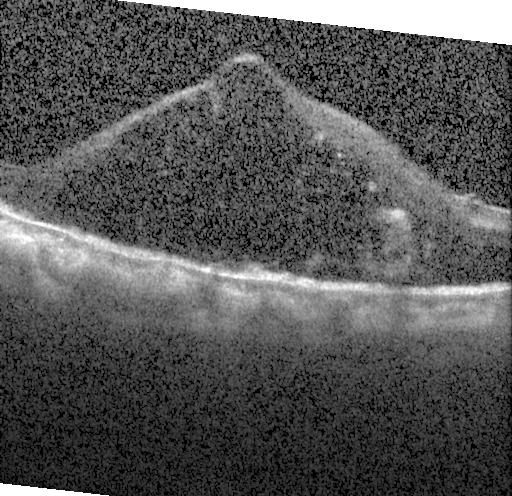 OCT B-scan; instrument: Heidelberg Spectralis; spectral-domain optical coherence tomography
Macular OCT: DME.